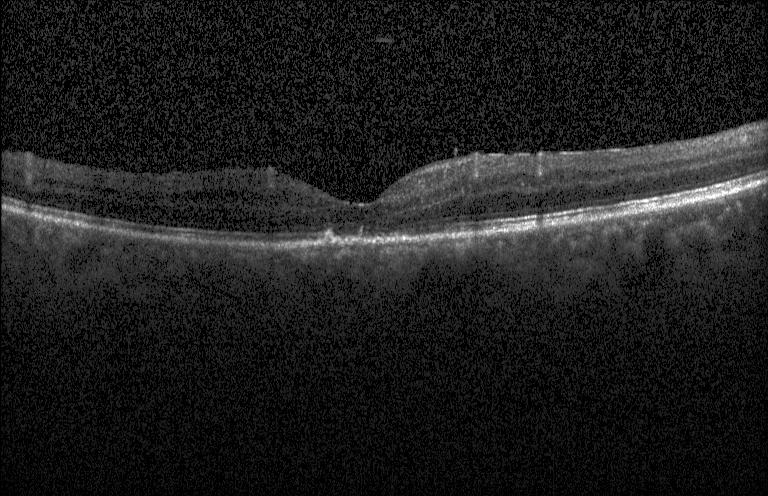
Instrument: Heidelberg Spectralis. Centered on the fovea. Retinal OCT B-scan. Spectral-domain OCT.
Multiple drusen.